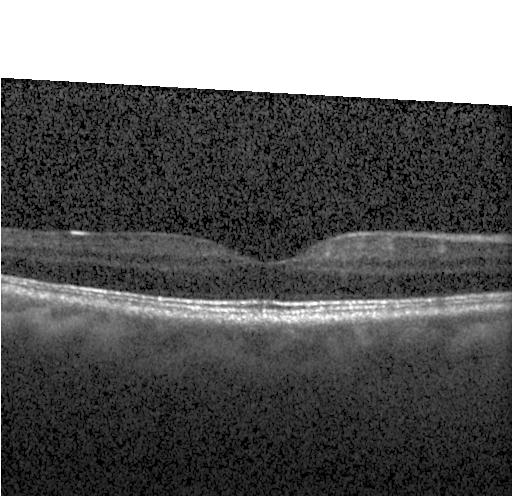
Finding: no evidence of choroidal neovascularization, diabetic macular edema, or drusen.